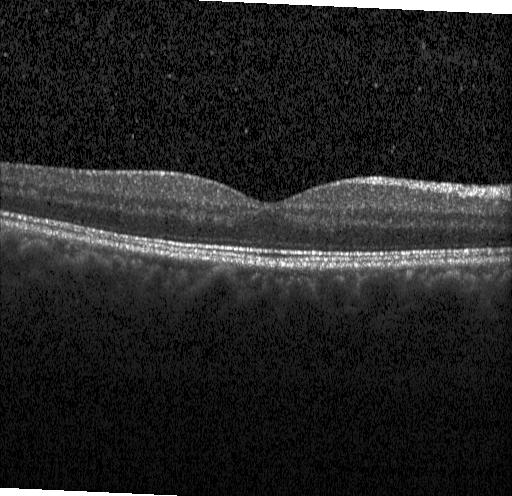
Fovea-centered; Heidelberg Spectralis OCT system; retinal OCT B-scan; SD-OCT — Diagnosis: no CNV, DME, or drusen.